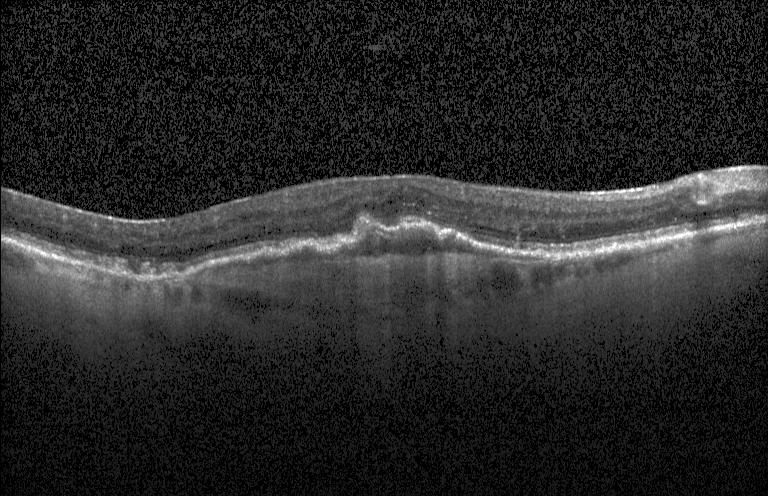

Dx: a choroidal neovascular membrane.